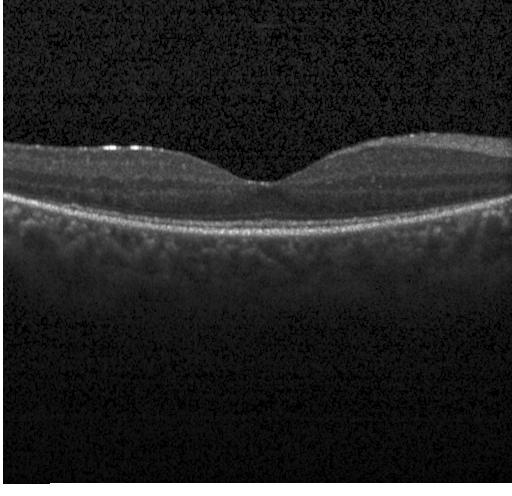 SD-OCT; retinal OCT cross-section
OCT finding: neither choroidal neovascularization, diabetic macular edema, nor drusen.